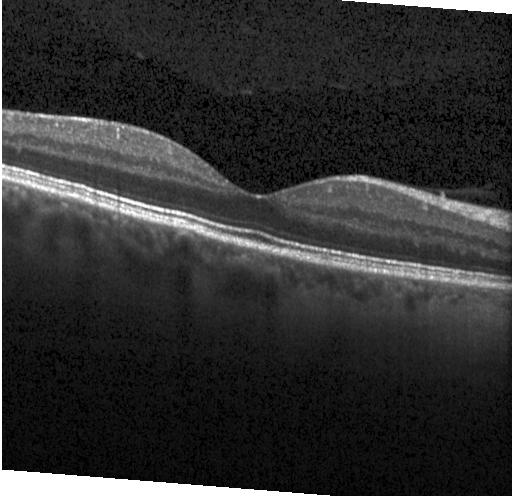 Assessment: no evidence of choroidal neovascularization, diabetic macular edema, or drusen.